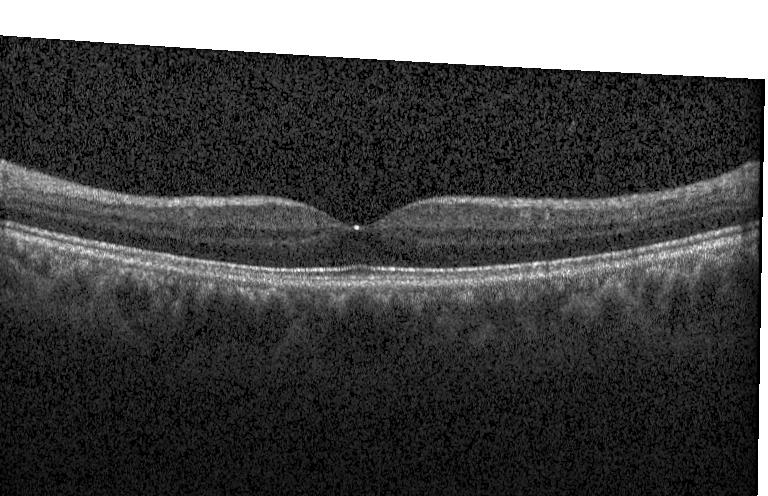
Spectral-domain optical coherence tomography, through the macula, OCT B-scan.
The scan shows no choroidal neovascularization, no diabetic macular edema, and no drusen.